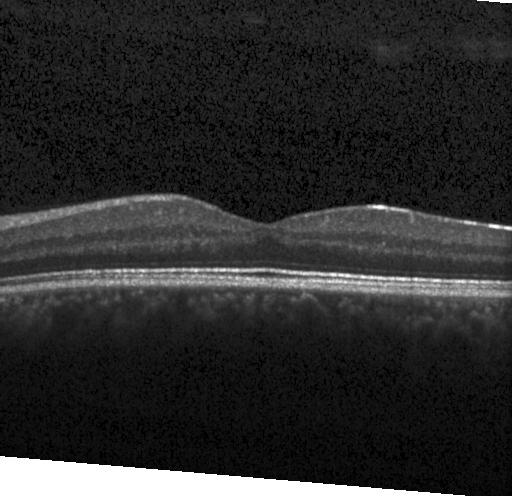

Optical coherence tomography scan.
OCT finding: no evidence of choroidal neovascularization, diabetic macular edema, or drusen.